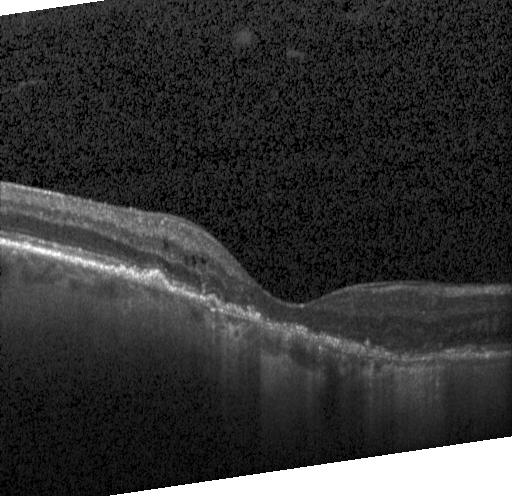 Optical coherence tomography B-scan — Assessment: choroidal neovascularization.